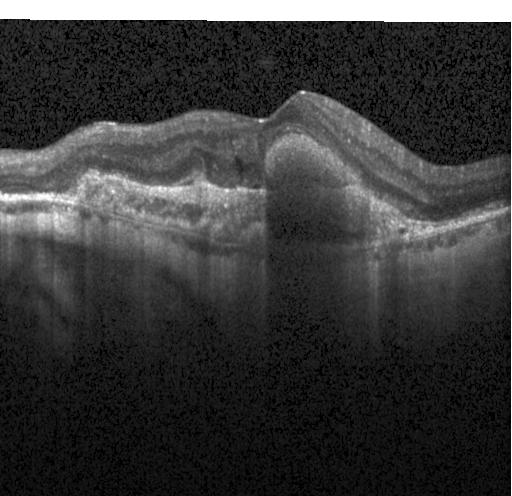

Finding: a choroidal neovascular membrane.